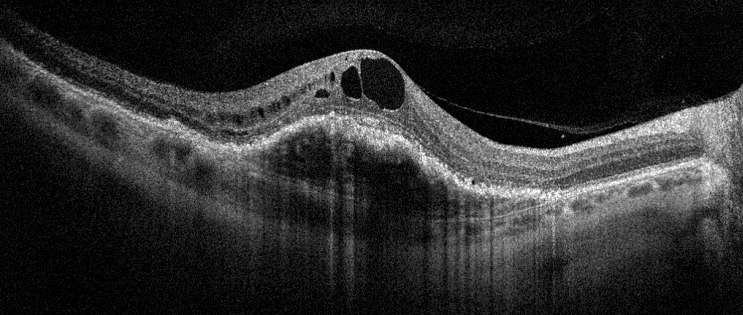

Fovea-centered, optical coherence tomography B-scan, right eye.
Diagnosis: age-related macular degeneration.